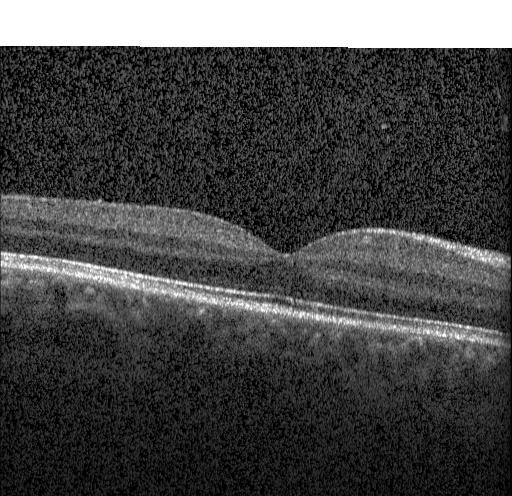 Instrument: Heidelberg Spectralis · spectral-domain optical coherence tomography · retinal OCT B-scan.
Dx: no CNV, DME, or drusen.